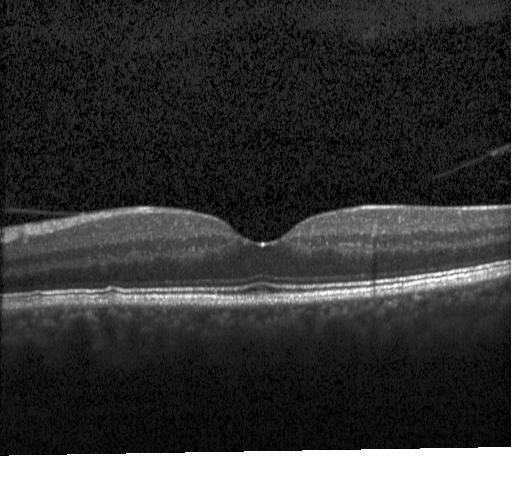

Optical coherence tomography scan; spectral-domain OCT.
No choroidal neovascularization, diabetic macular edema, or drusen.